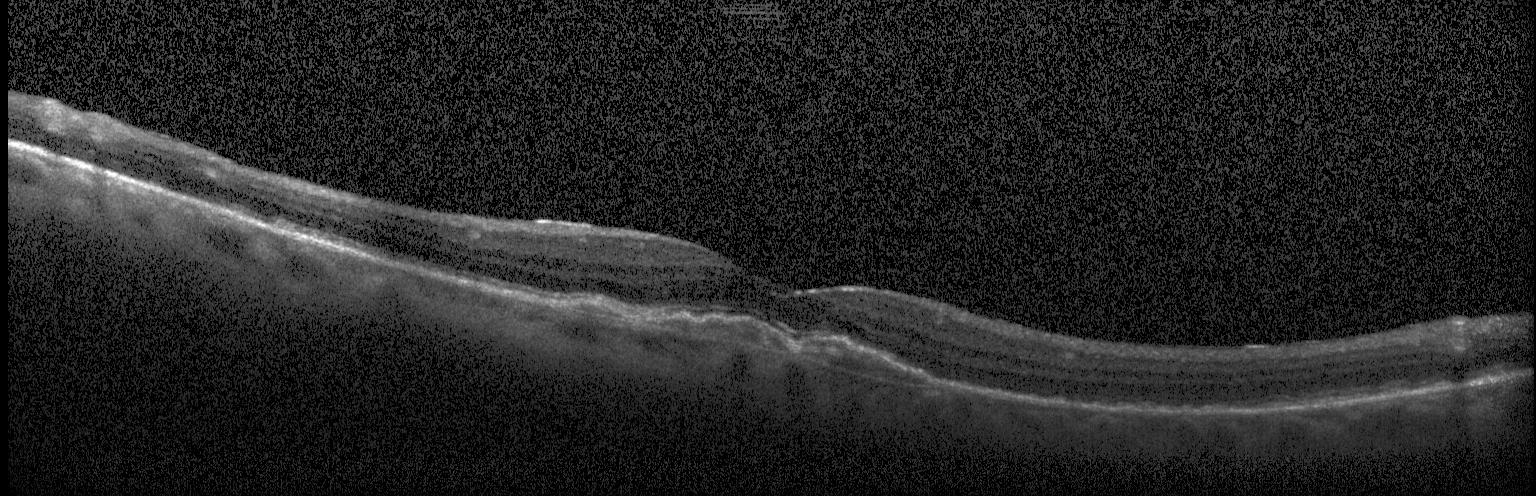

Macular OCT: a choroidal neovascular membrane.